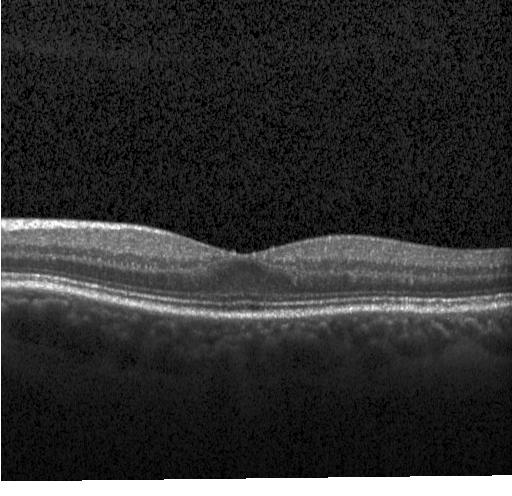 Macular OCT demonstrating no evidence of choroidal neovascularization, diabetic macular edema, or drusen.